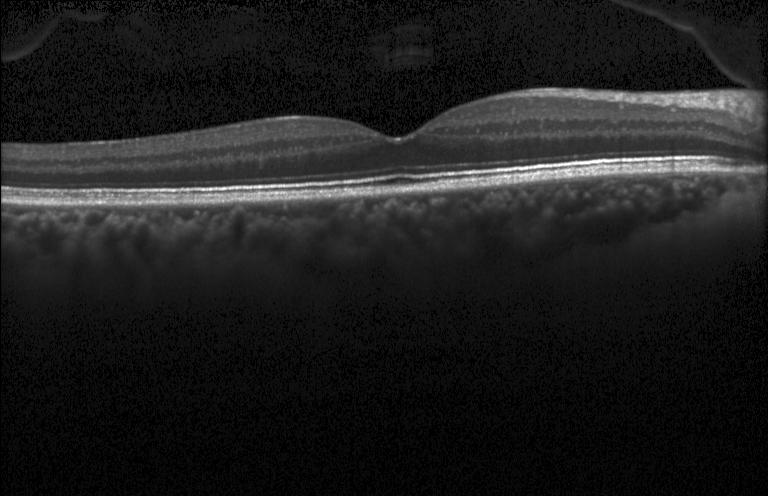

Spectral-domain optical coherence tomography; retinal OCT cross-section. The scan shows no choroidal neovascularization, diabetic macular edema, or drusen.